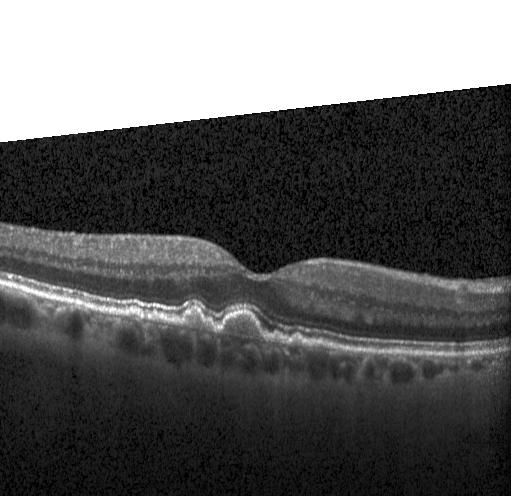

OCT B-scan showing drusen.